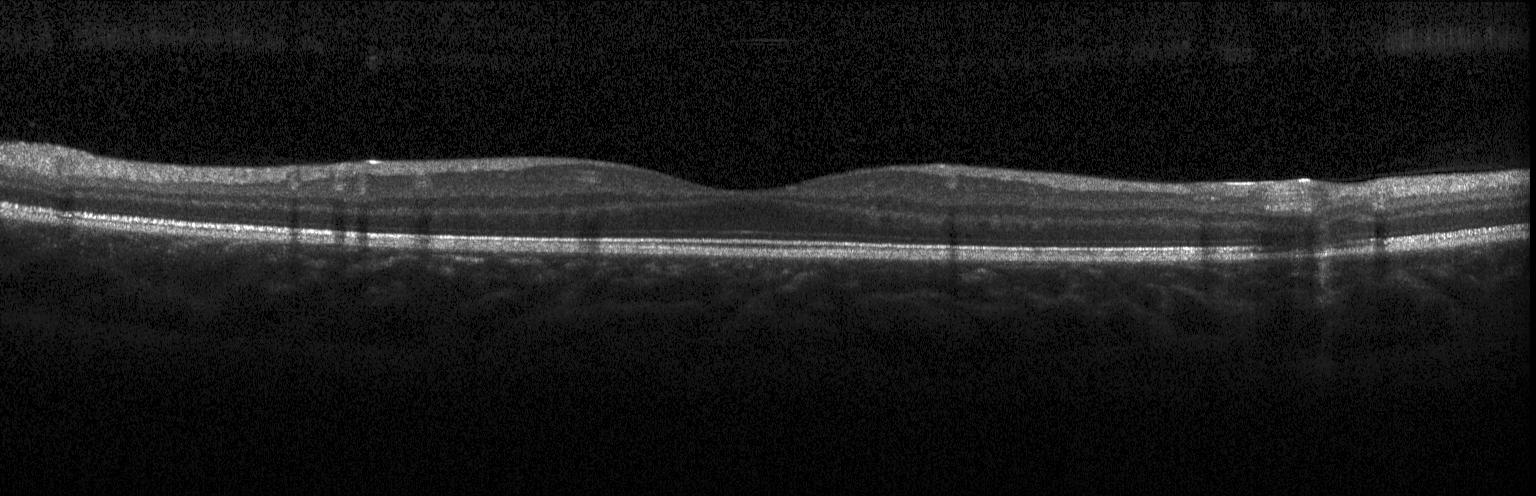

Macular OCT demonstrating no evidence of choroidal neovascularization, diabetic macular edema, or drusen.